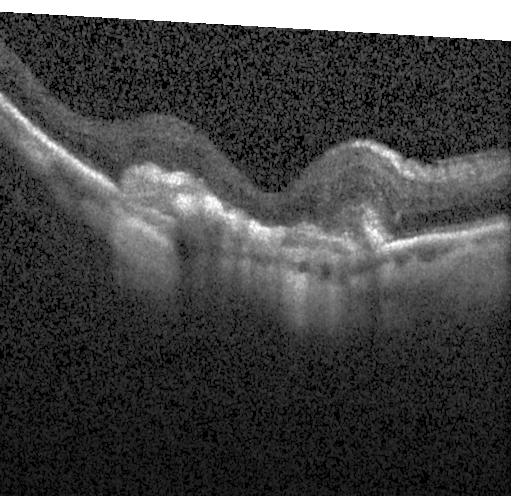

OCT B-scan showing a choroidal neovascular membrane.